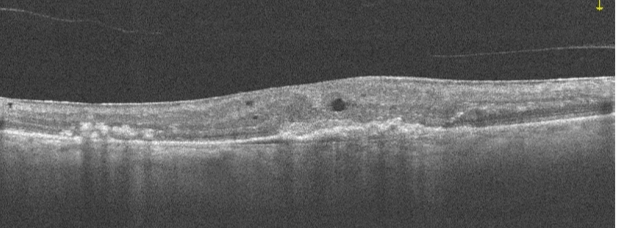
Macular scan; OCT line scan — The scan shows age-related macular degeneration (AMD).